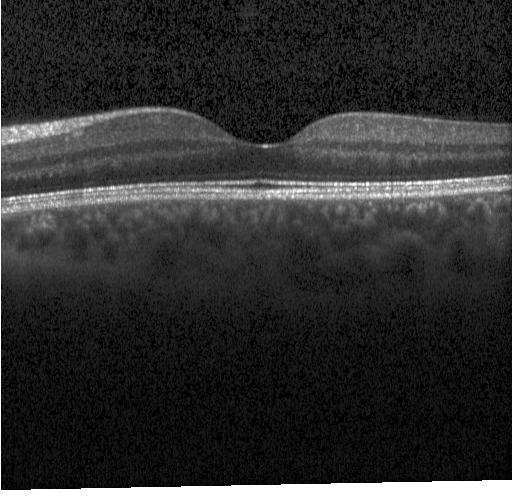
Spectral-domain OCT, OCT B-scan, acquired on a Heidelberg Spectralis.
Impression: no choroidal neovascularization, diabetic macular edema, or drusen.